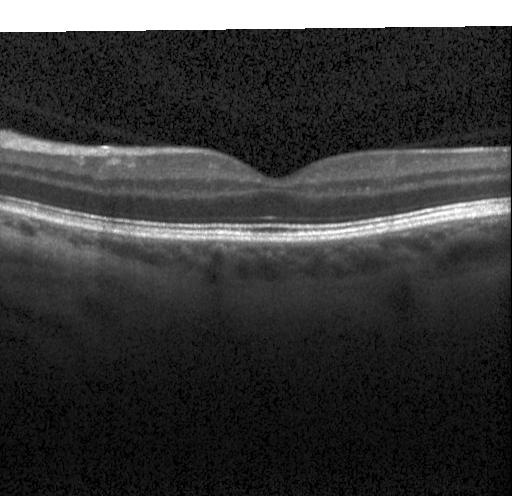

OCT B-scan showing no evidence of CNV, DME, or drusen.